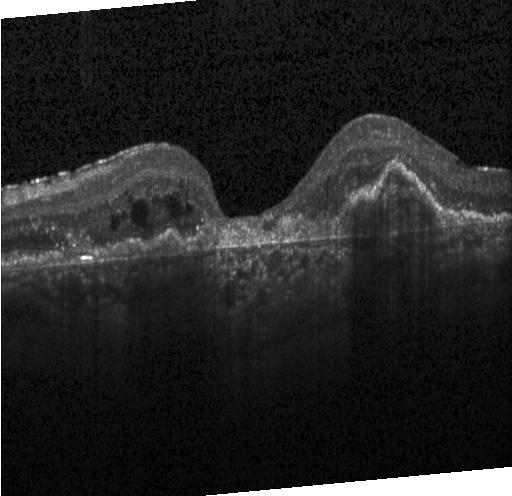
Spectral-domain OCT; instrument: Heidelberg Spectralis; retinal OCT cross-section; fovea-centered
This B-scan demonstrates a choroidal neovascular membrane.